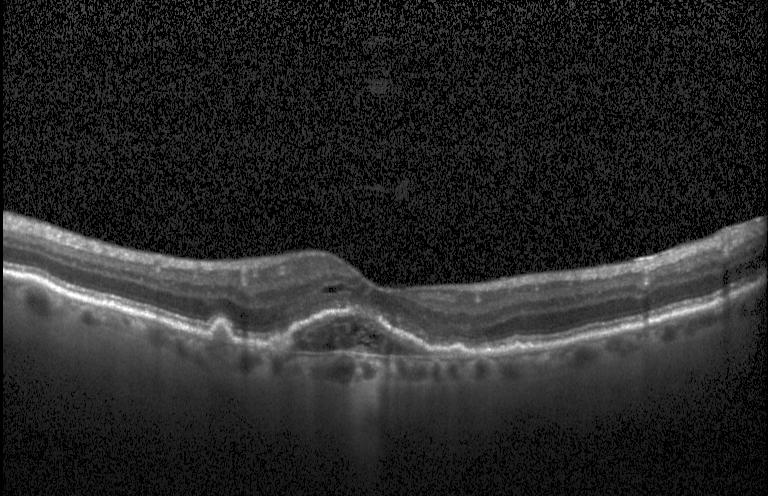
Spectral-domain OCT, centered on the fovea, retinal OCT cross-section.
Assessment: choroidal neovascularization (CNV).